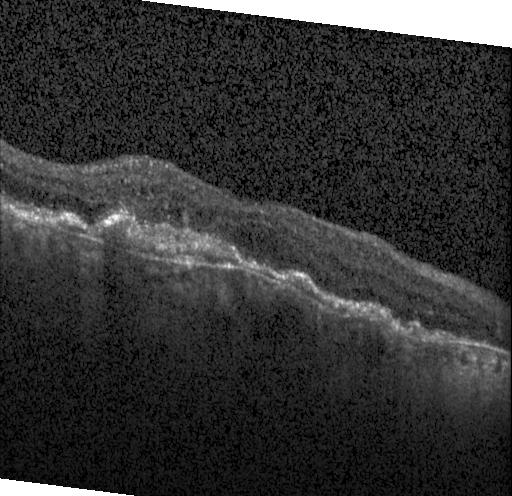
OCT line scan
Finding: a choroidal neovascular membrane.